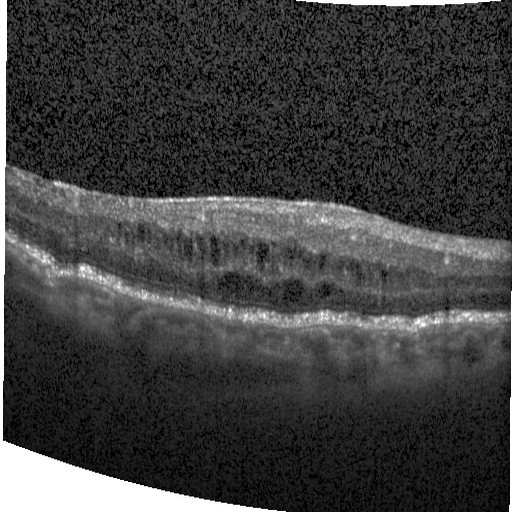 Macular OCT demonstrating diabetic macular edema (DME).